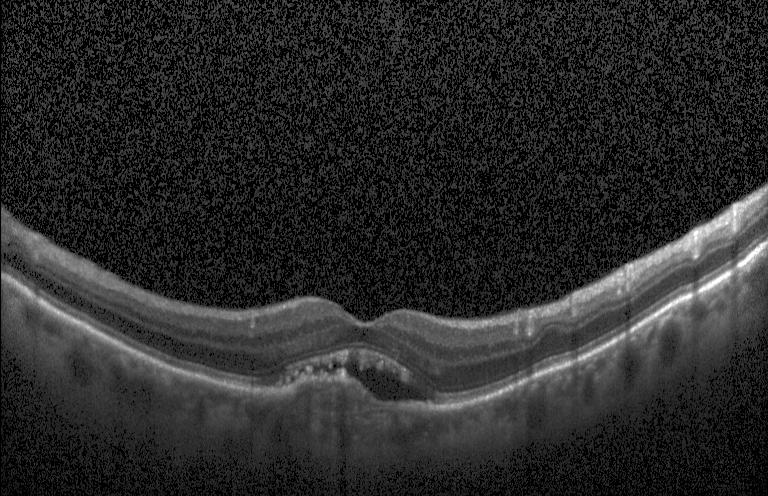 Centered on the fovea · OCT line scan · spectral-domain optical coherence tomography.
Assessment: a choroidal neovascular membrane.